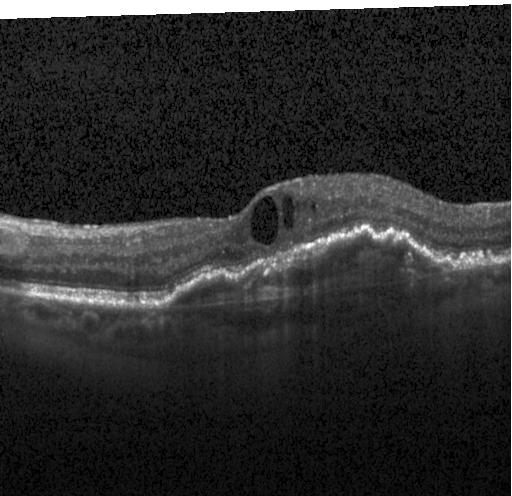
Spectral-domain optical coherence tomography, optical coherence tomography B-scan. Finding: a choroidal neovascular membrane.